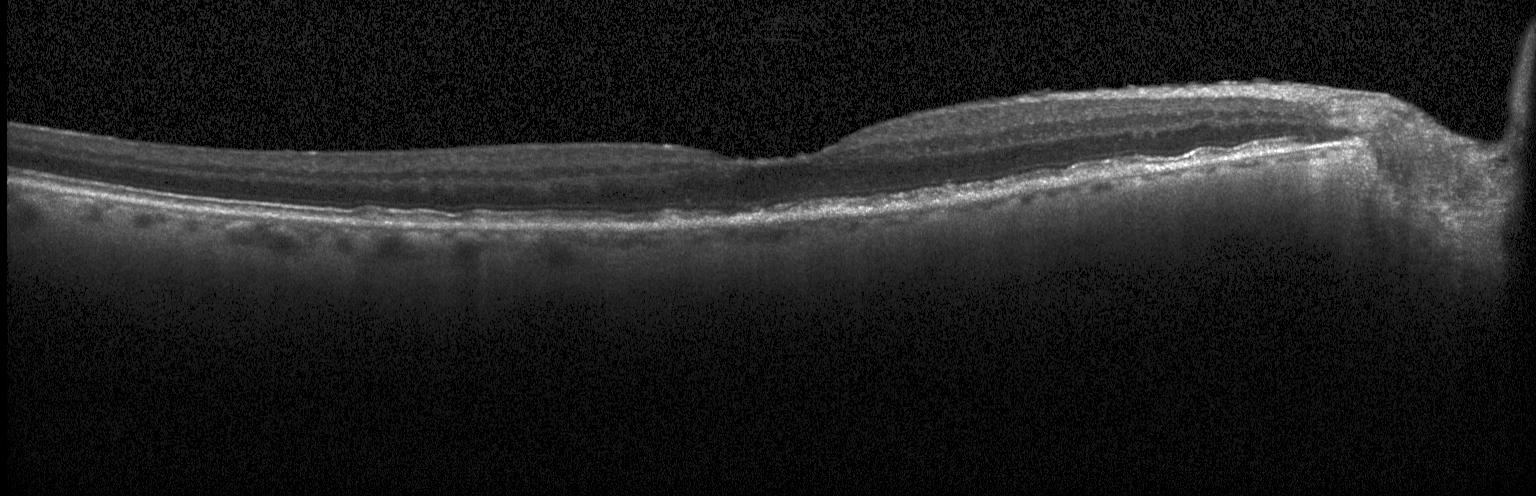 The scan shows sub-RPE drusenoid deposits.